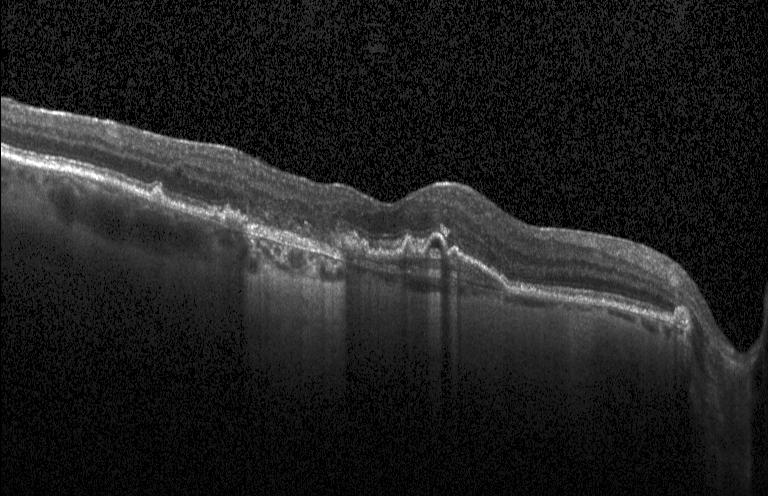

Macular scan; optical coherence tomography B-scan.
Finding: a choroidal neovascular membrane.